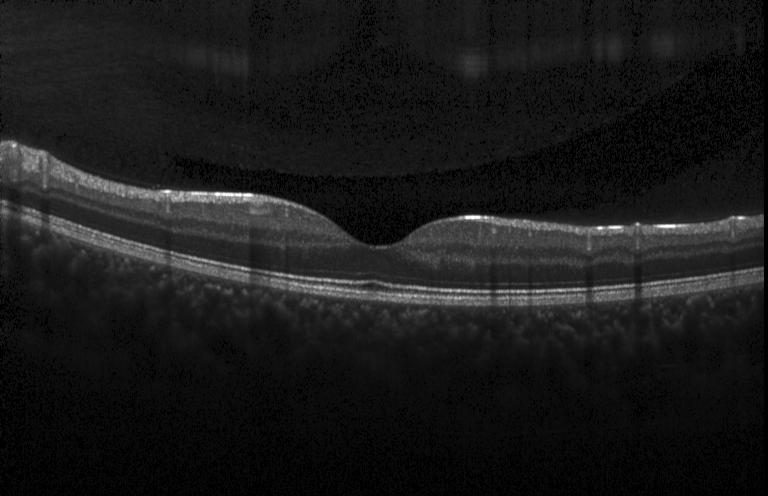
Horizontal scan through the fovea. Optical coherence tomography B-scan — Neither choroidal neovascularization, diabetic macular edema, nor drusen.